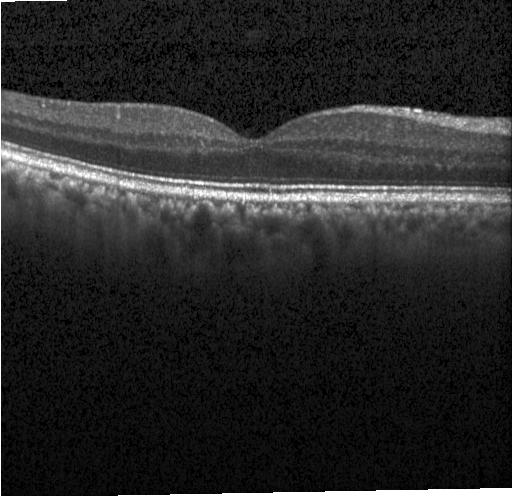
Retinal OCT cross-section showing no CNV, DME, or drusen.